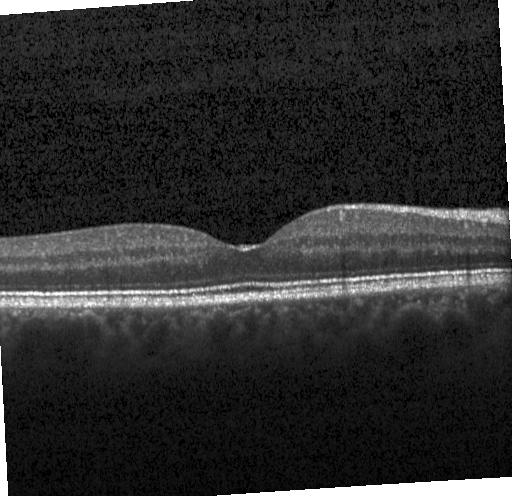

Heidelberg Spectralis OCT system. Optical coherence tomography scan. Fovea-centered.
Impression: neither CNV, DME, nor drusen.